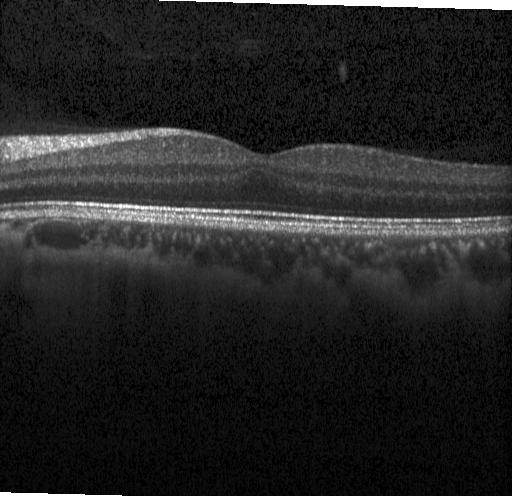
Macular OCT demonstrating no evidence of choroidal neovascularization, diabetic macular edema, or drusen.